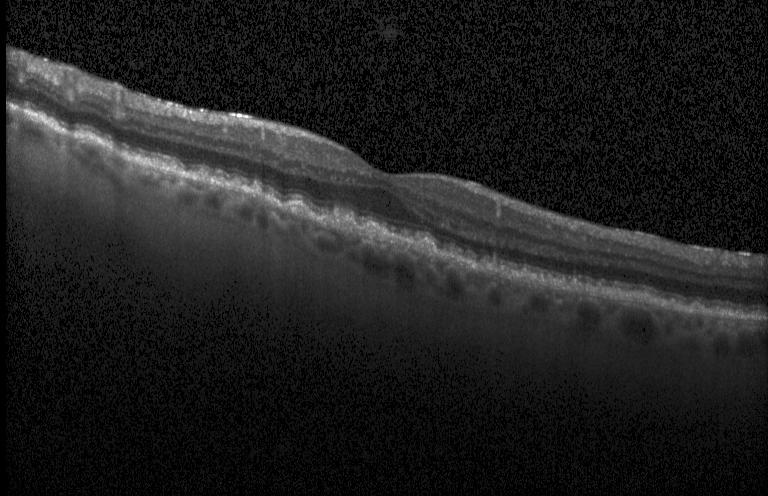

Retinal OCT cross-section
Finding: sub-RPE drusenoid deposits.